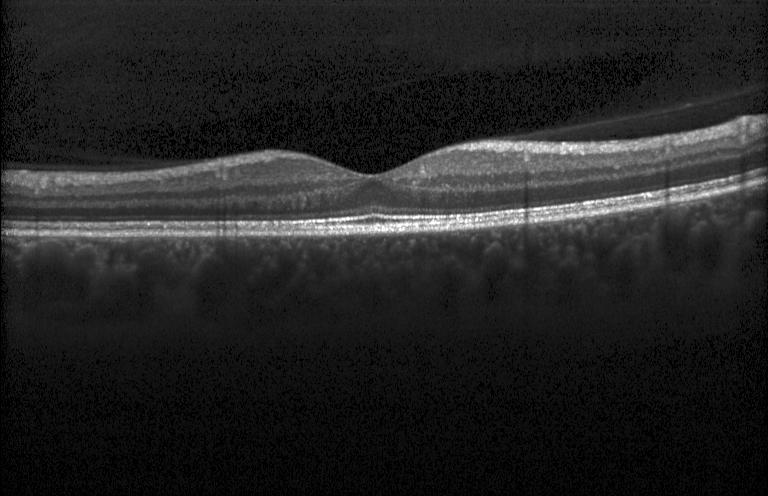
OCT line scan — This B-scan demonstrates no choroidal neovascularization, diabetic macular edema, or drusen.